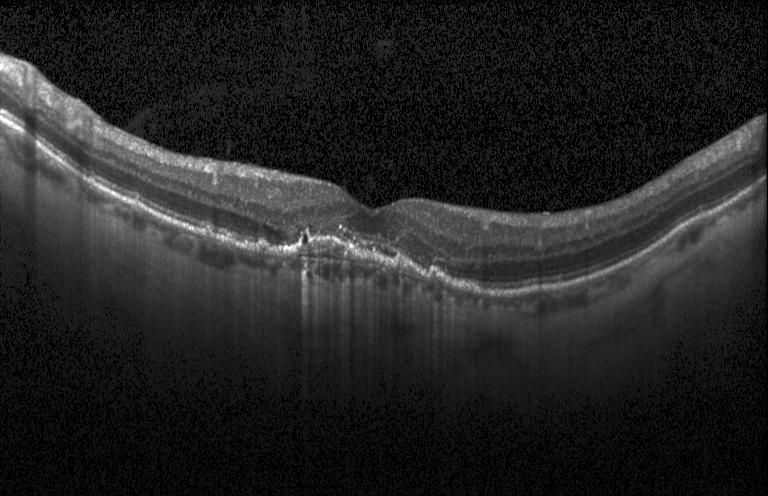

Instrument: Heidelberg Spectralis, SD-OCT, optical coherence tomography B-scan.
Diagnosis: choroidal neovascularization (CNV).